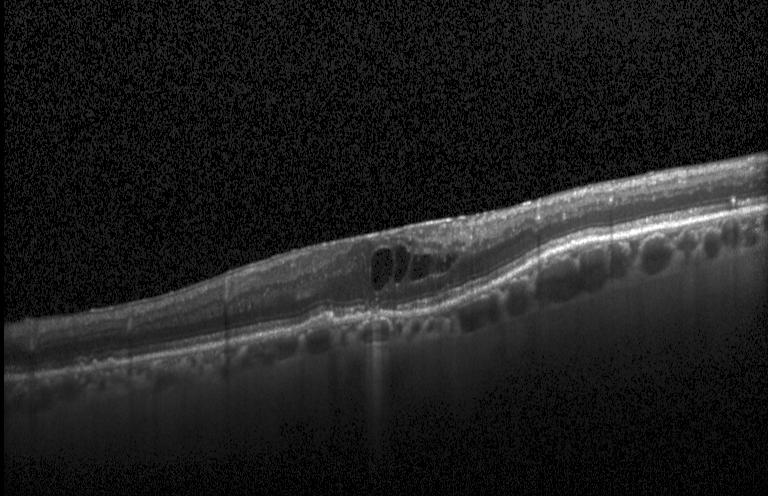 Dx: choroidal neovascularization (CNV).